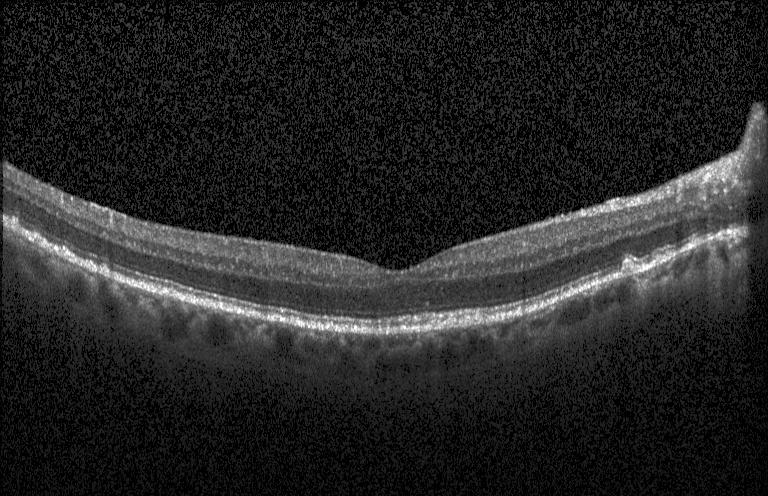
OCT B-scan — This B-scan demonstrates drusen.